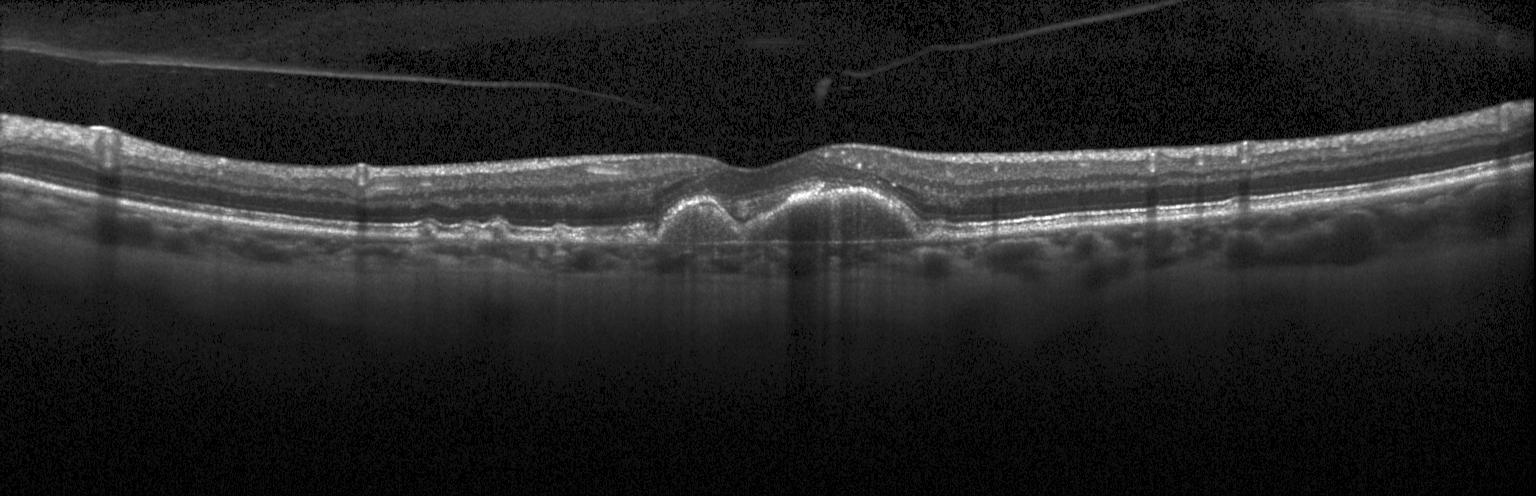 Retinal OCT B-scan.
A choroidal neovascular membrane.